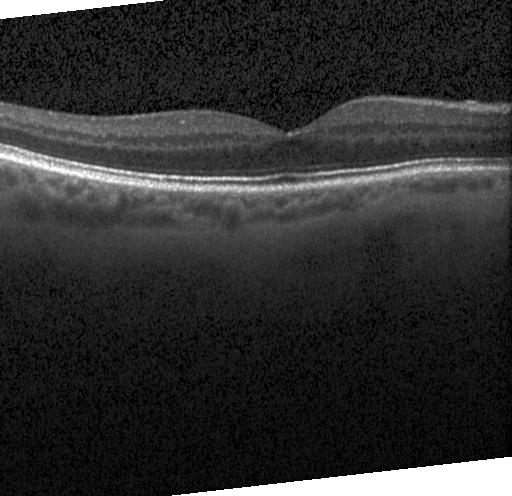 Optical coherence tomography B-scan; fovea-centered; acquired on a Heidelberg Spectralis
This B-scan demonstrates no evidence of choroidal neovascularization, diabetic macular edema, or drusen.